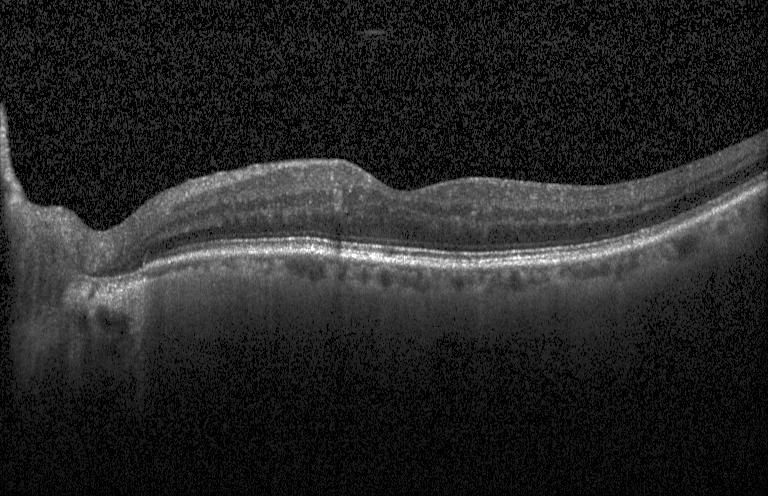
SD-OCT. Retinal OCT cross-section. Heidelberg Spectralis.
OCT finding: no evidence of choroidal neovascularization, diabetic macular edema, or drusen.